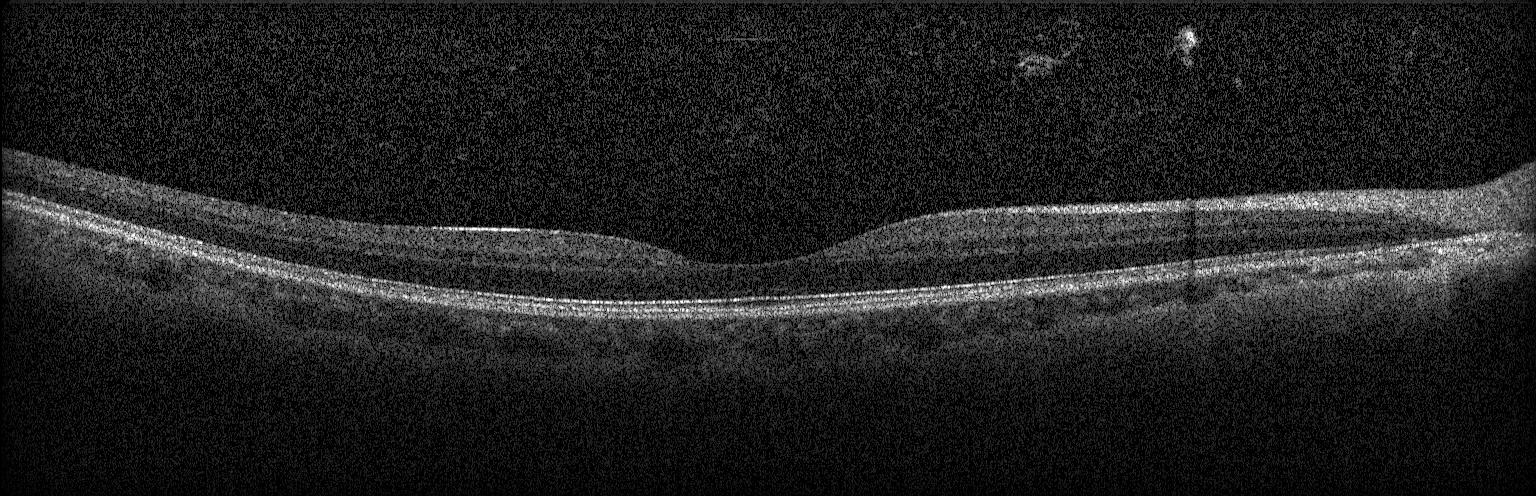 Optical coherence tomography scan; spectral-domain optical coherence tomography; through the macula; Heidelberg Spectralis.
Macular OCT: no CNV, DME, or drusen.